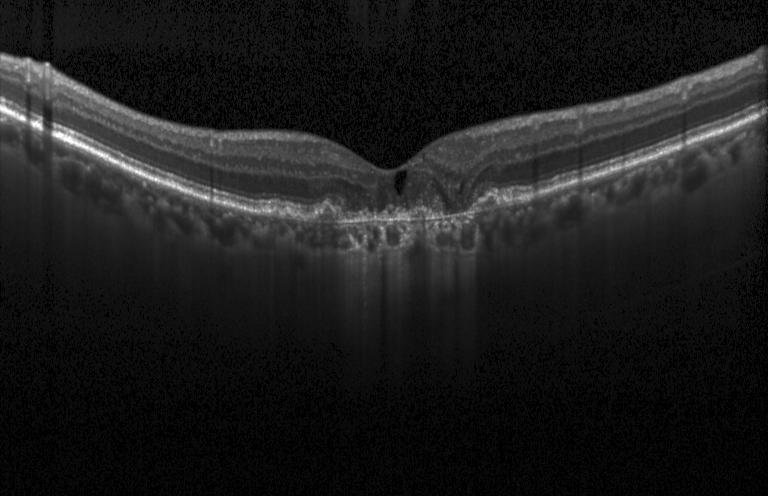
Heidelberg Spectralis, spectral-domain optical coherence tomography, retinal OCT B-scan, horizontal scan through the fovea
Diagnosis: CNV.